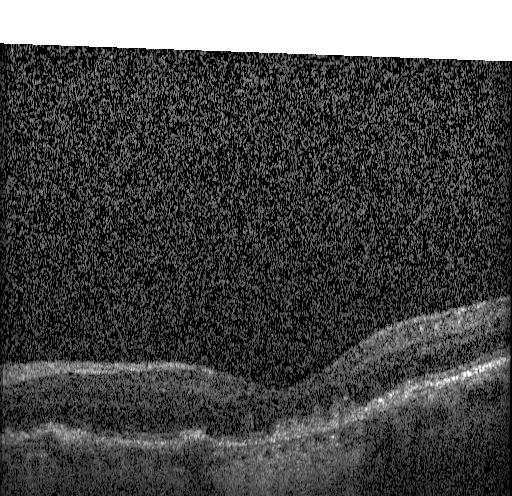 OCT finding: a choroidal neovascular membrane.